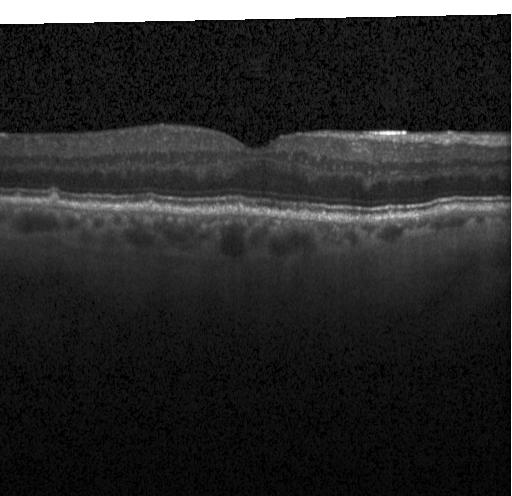
Macular OCT demonstrating drusen.